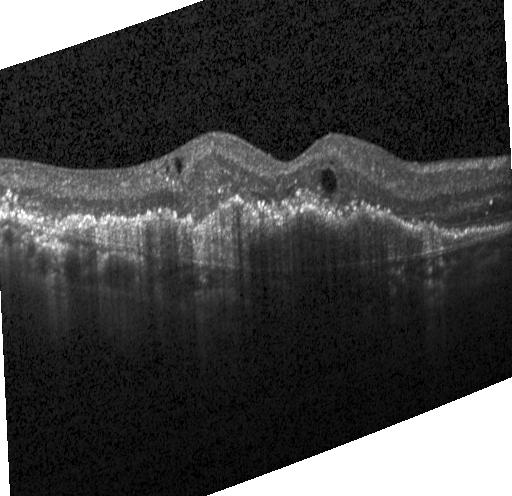

Dx: choroidal neovascularization (CNV).